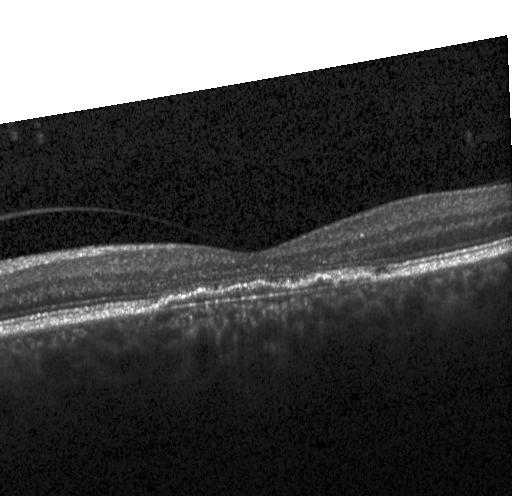 Macular OCT demonstrating a choroidal neovascular membrane.